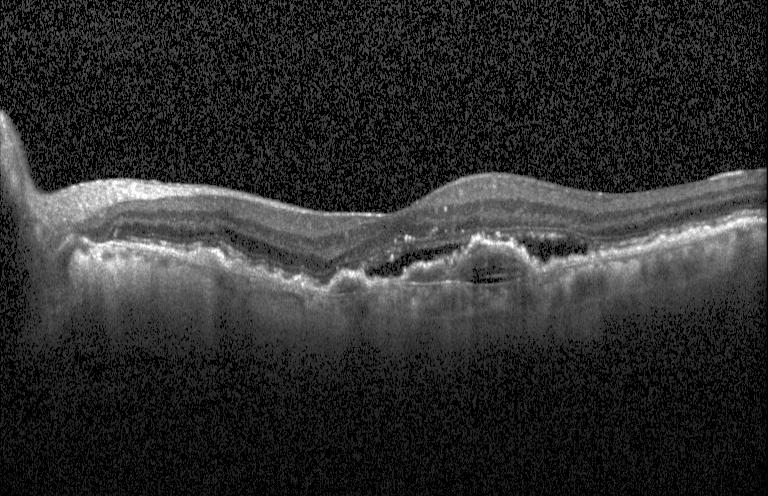

Retinal OCT B-scan
Macular OCT: choroidal neovascularization.